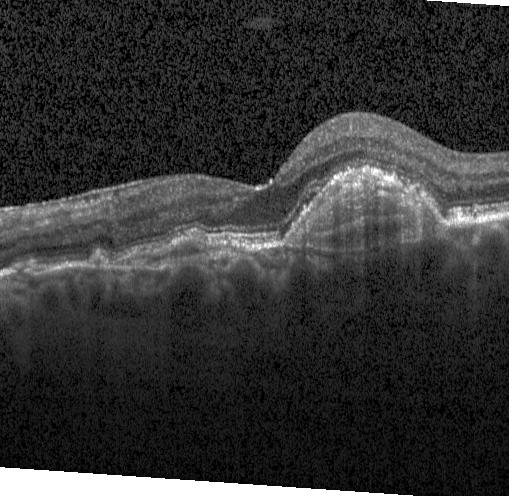
OCT B-scan — The scan shows CNV.